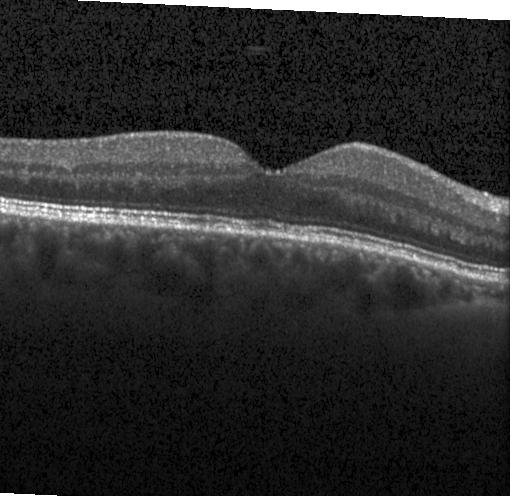 Macular OCT: no CNV, no DME, and no drusen.